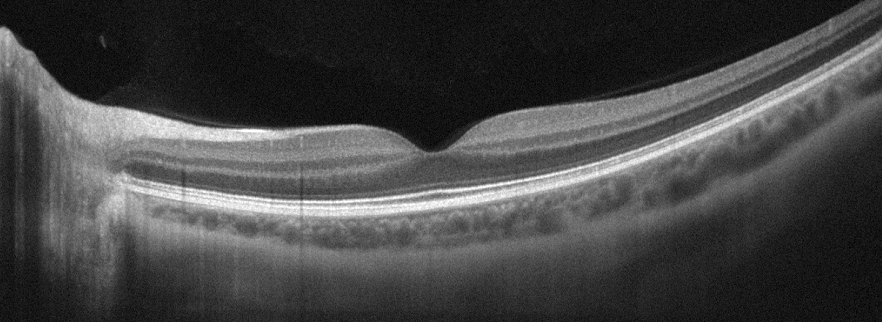

Right eye; retinal OCT cross-section.
Macular OCT: no AMD, DME, ERM, RAO, RVO, or VID.